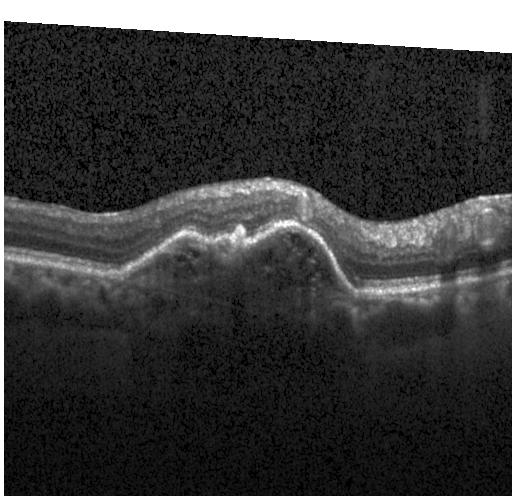 Through the macula. OCT line scan. Spectral-domain optical coherence tomography. Instrument: Heidelberg Spectralis — Dx: choroidal neovascularization (CNV).